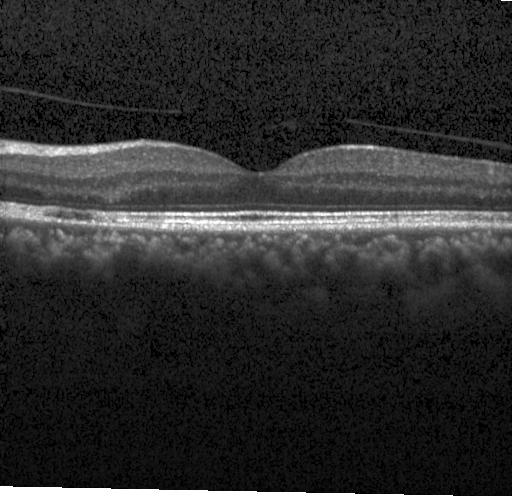 Horizontal scan through the fovea. Heidelberg Spectralis OCT system. Retinal OCT cross-section
Dx: neither CNV, DME, nor drusen.